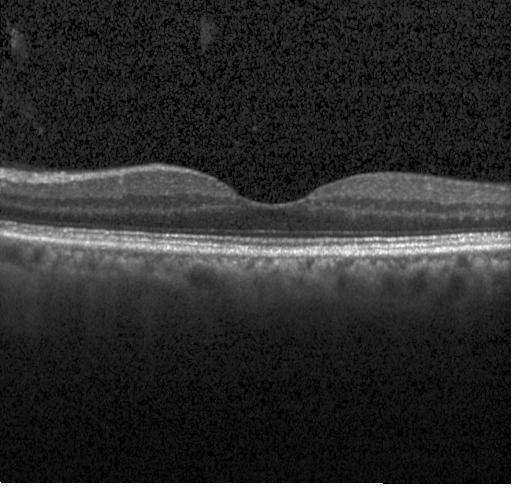
OCT B-scan.
Diagnosis: no choroidal neovascularization, diabetic macular edema, or drusen.